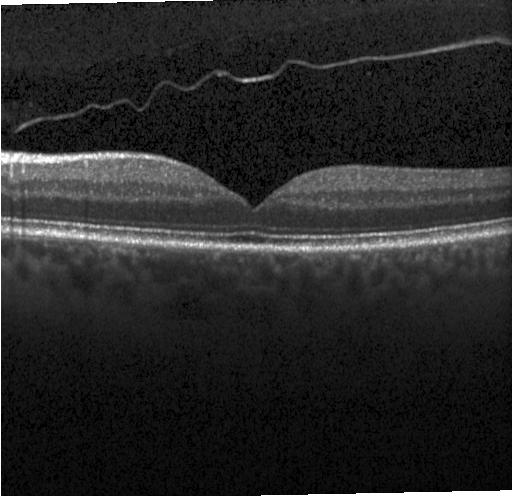 Heidelberg Spectralis OCT system, through the macula, optical coherence tomography B-scan, SD-OCT.
Diagnosis: no evidence of CNV, DME, or drusen.